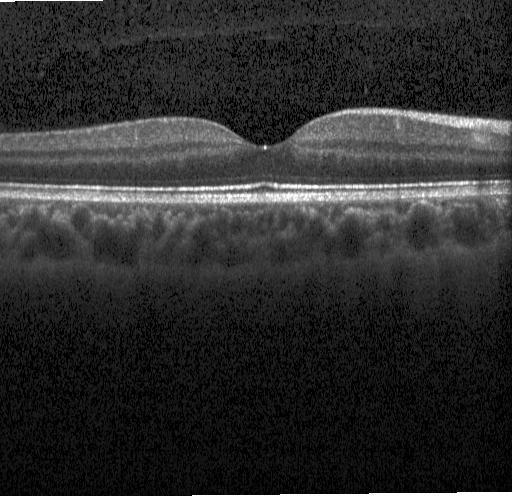
Macular OCT demonstrating no choroidal neovascularization, diabetic macular edema, or drusen.